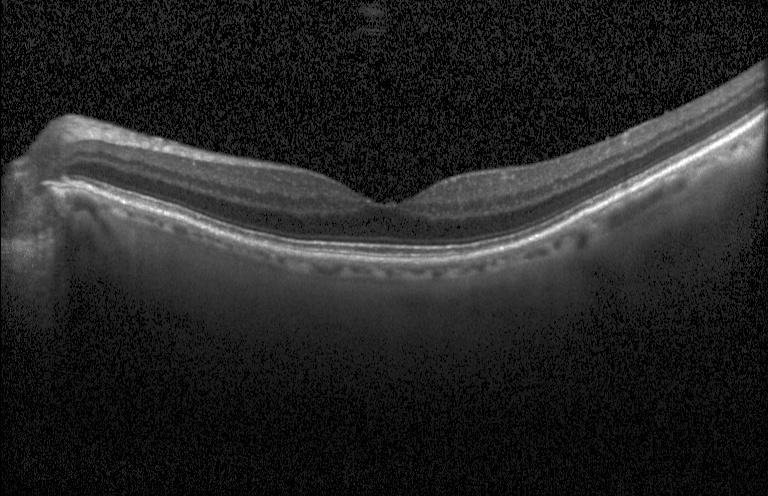
Retinal OCT cross-section · SD-OCT.
Assessment: neither choroidal neovascularization, diabetic macular edema, nor drusen.